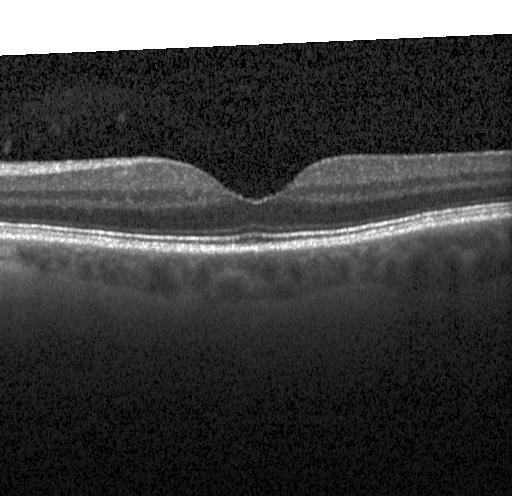

This B-scan demonstrates no evidence of CNV, DME, or drusen.